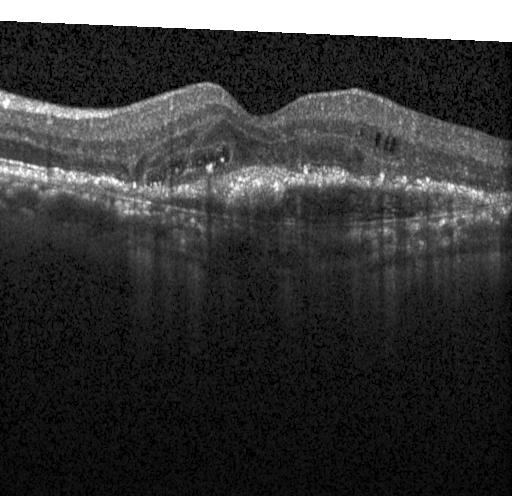

Heidelberg Spectralis OCT system, OCT B-scan, SD-OCT. OCT finding: a choroidal neovascular membrane.